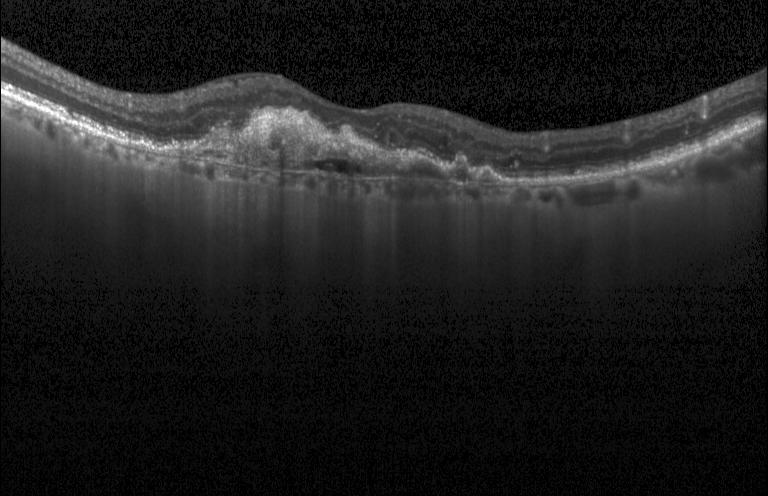
Impression: a choroidal neovascular membrane.